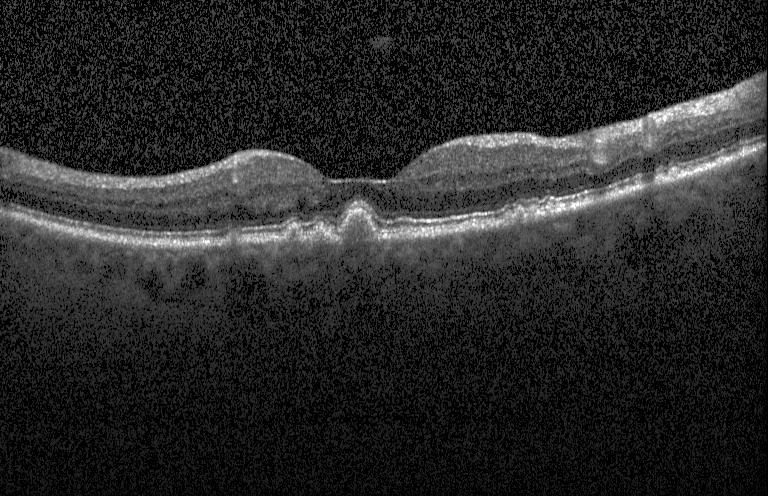

Finding: sub-RPE drusenoid deposits.